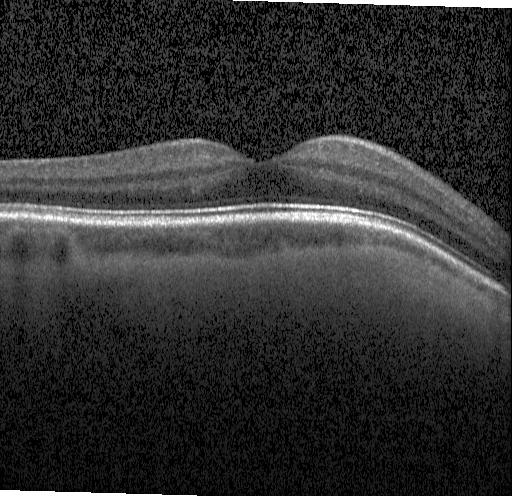
Impression: neither choroidal neovascularization, diabetic macular edema, nor drusen.